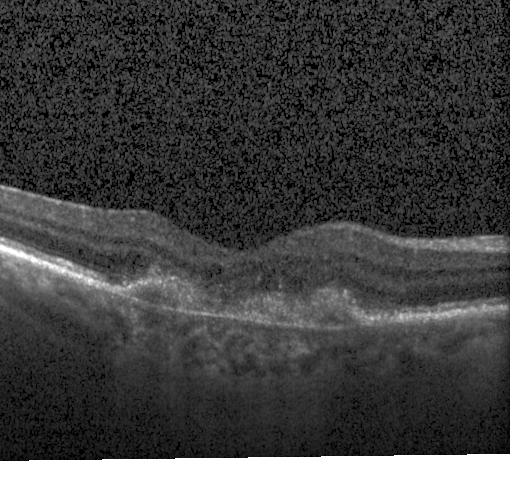

Fovea-centered, OCT B-scan — OCT finding: a choroidal neovascular membrane.